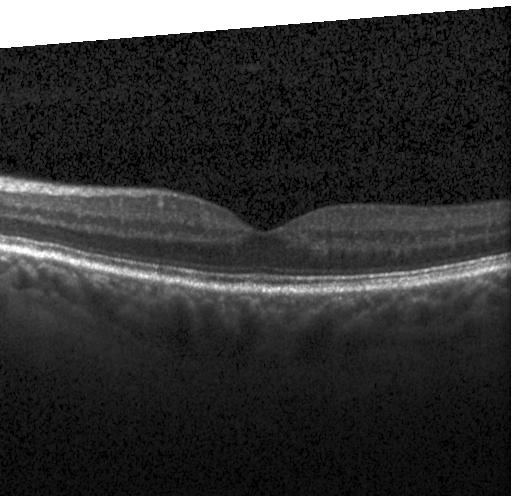
Finding: no evidence of CNV, DME, or drusen.